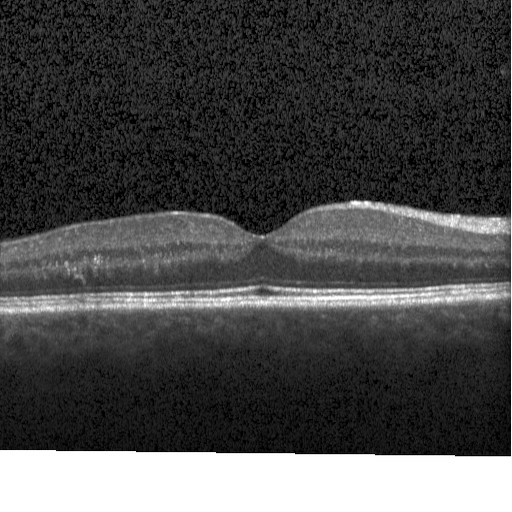
Impression: DME.